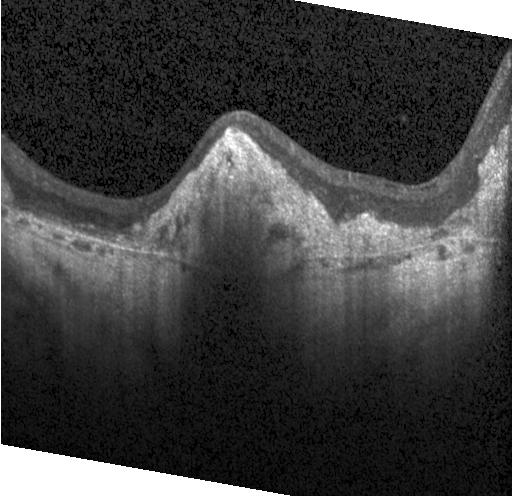

Instrument: Heidelberg Spectralis; spectral-domain OCT; retinal OCT cross-section; fovea-centered — Diagnosis: choroidal neovascularization.